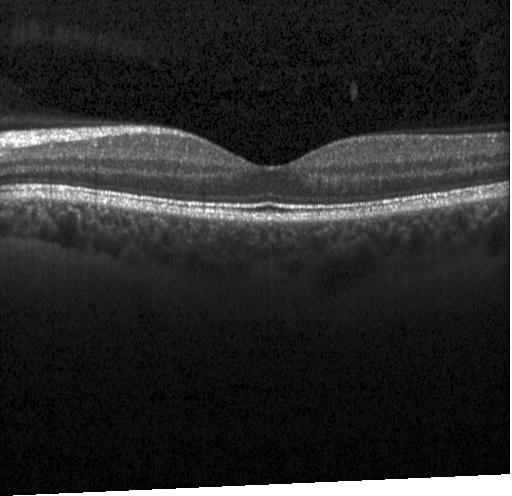
Through the macula, retinal OCT cross-section — OCT finding: no evidence of choroidal neovascularization, diabetic macular edema, or drusen.